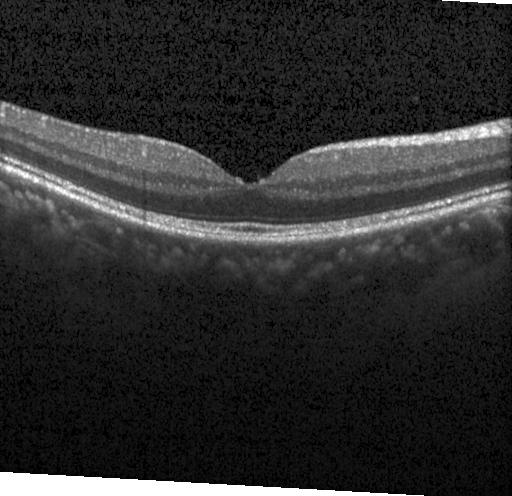

Macular OCT: no choroidal neovascularization, diabetic macular edema, or drusen.